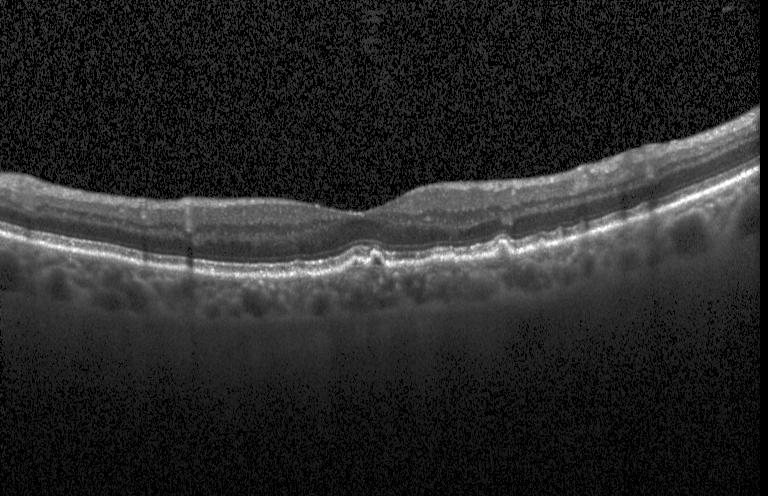

Spectral-domain optical coherence tomography · horizontal scan through the fovea · retinal OCT B-scan. Macular OCT: sub-RPE drusenoid deposits.